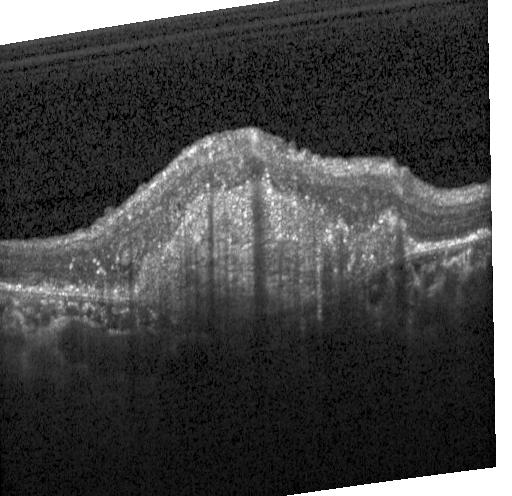
Horizontal scan through the fovea; spectral-domain OCT; acquired on a Heidelberg Spectralis; optical coherence tomography scan
A choroidal neovascular membrane.